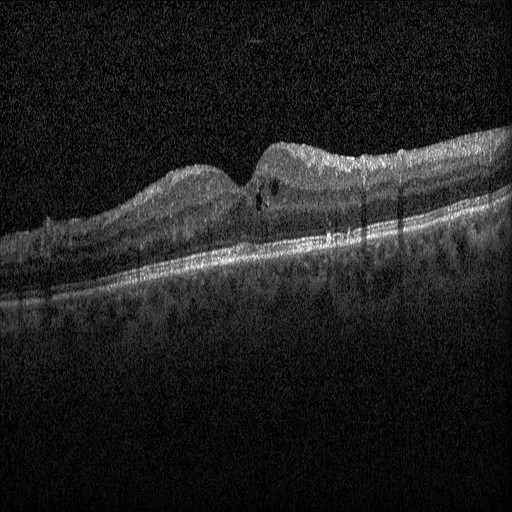 This B-scan demonstrates diabetic macular edema.